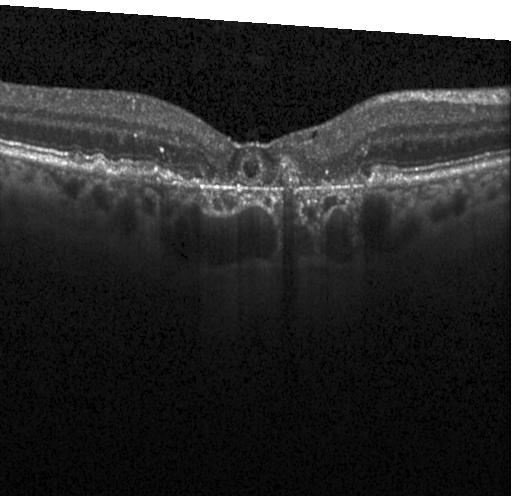
Optical coherence tomography B-scan. Assessment: choroidal neovascularization.